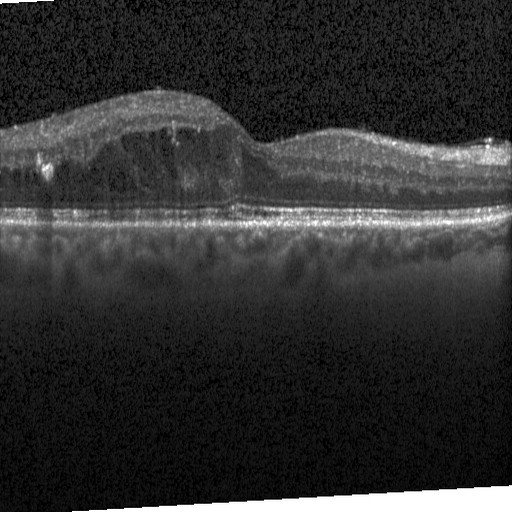 Acquired on a Heidelberg Spectralis · macular scan · spectral-domain OCT · OCT line scan
The scan shows diabetic macular edema.